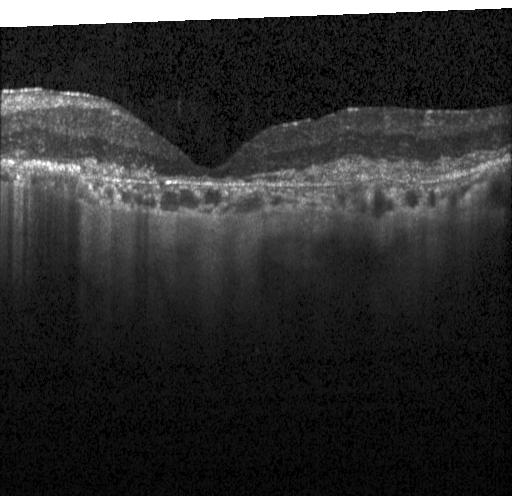
Retinal OCT B-scan; Heidelberg Spectralis OCT system; spectral-domain optical coherence tomography.
Diagnosis: CNV.